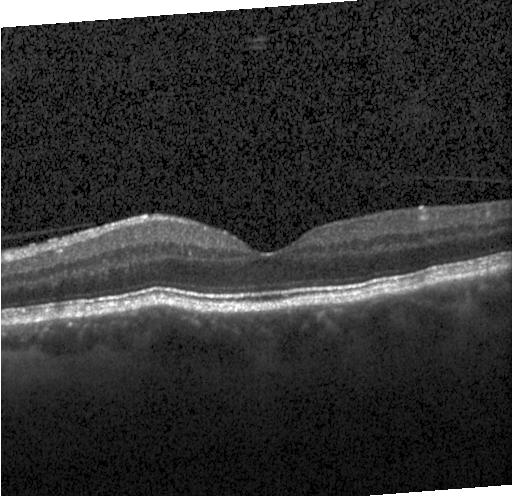 Optical coherence tomography scan, acquired on a Heidelberg Spectralis
Macular OCT: neither CNV, DME, nor drusen.